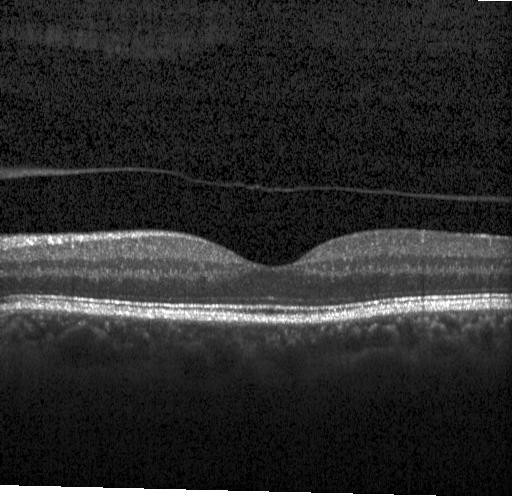 Optical coherence tomography B-scan
Macular OCT: no evidence of choroidal neovascularization, diabetic macular edema, or drusen.